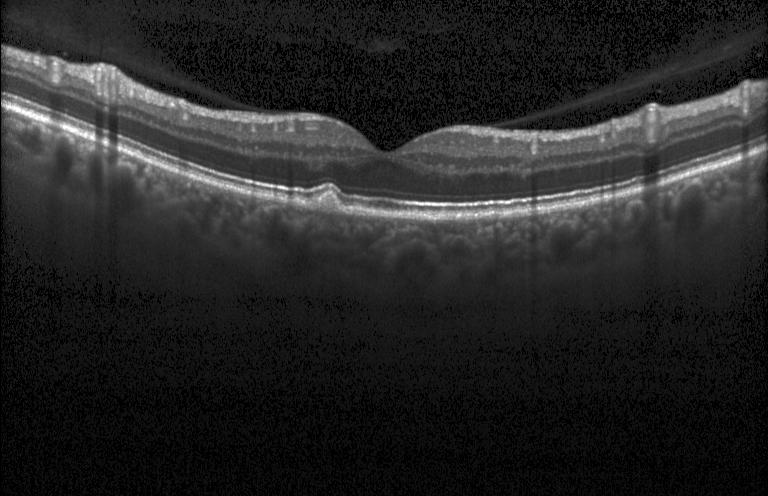
Retinal OCT cross-section showing sub-RPE drusenoid deposits.